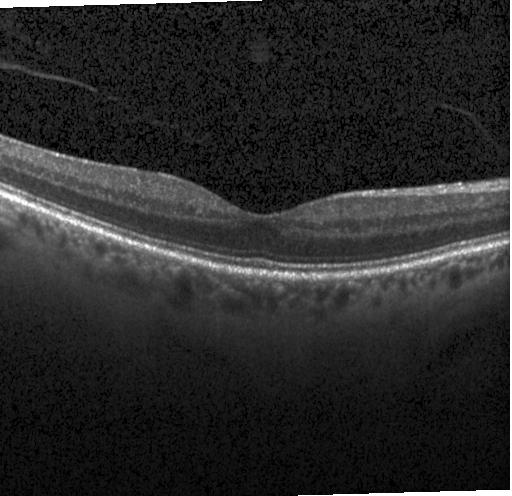 Finding: no choroidal neovascularization, diabetic macular edema, or drusen.